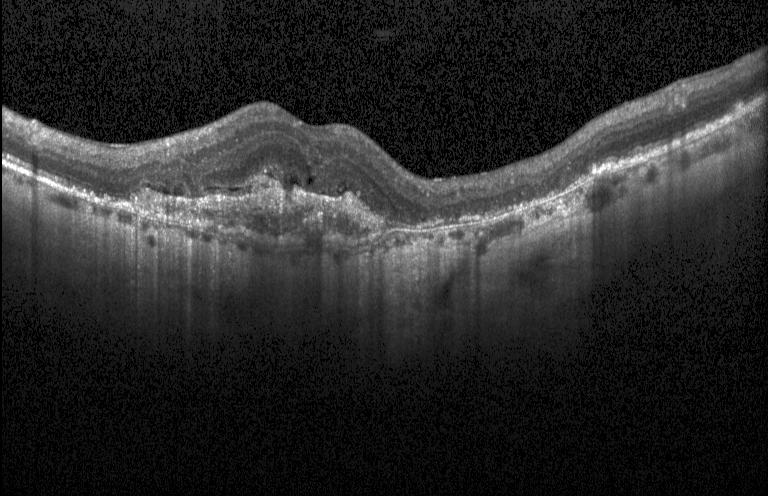
Optical coherence tomography scan. A choroidal neovascular membrane.